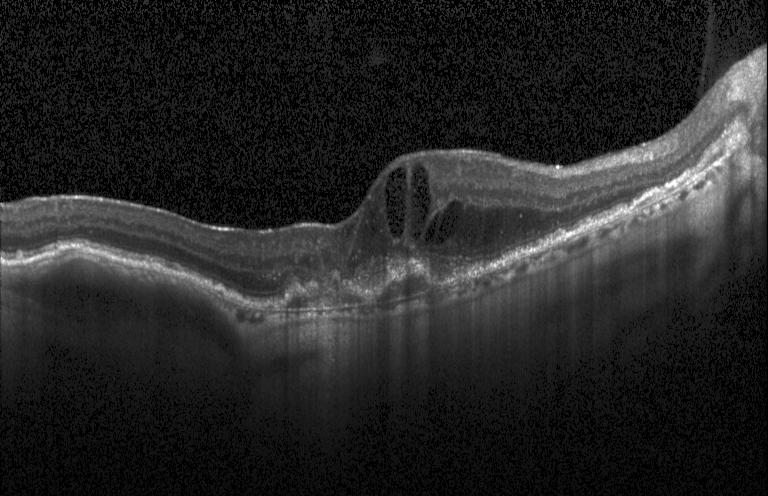

The scan shows a choroidal neovascular membrane.